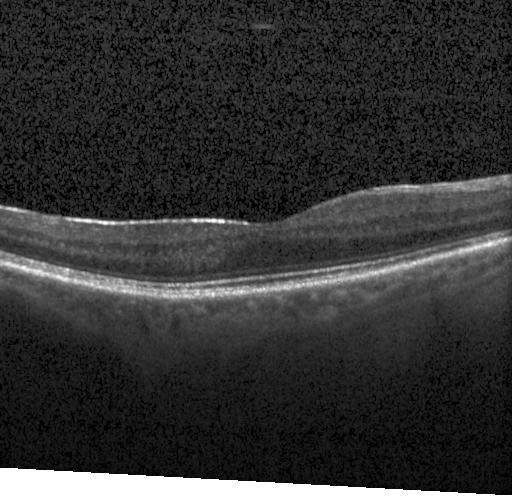 Retinal OCT B-scan. Impression: no evidence of CNV, DME, or drusen.